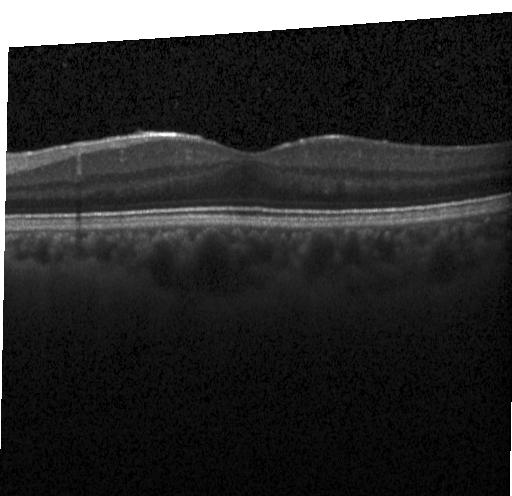 Instrument: Heidelberg Spectralis, optical coherence tomography scan, SD-OCT, macular scan.
Assessment: no CNV, DME, or drusen.